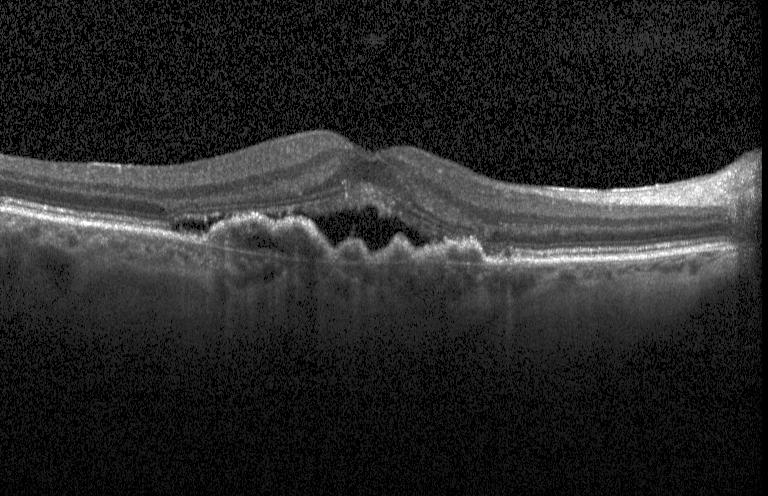

OCT B-scan showing a choroidal neovascular membrane.